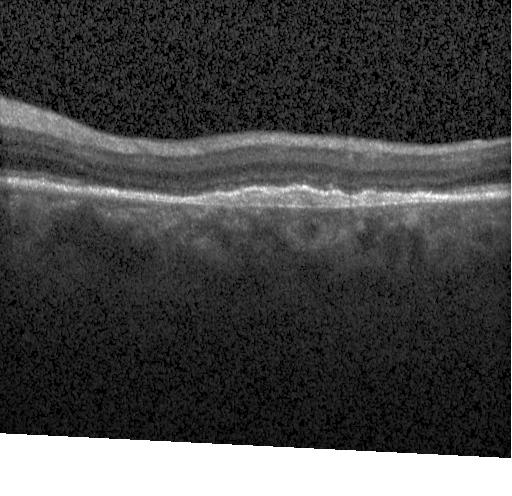
OCT B-scan.
Impression: a choroidal neovascular membrane.